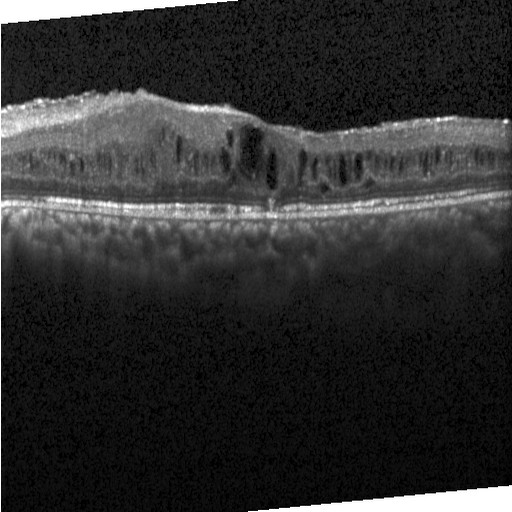 Heidelberg Spectralis. Through the macula. OCT B-scan — Diagnosis: diabetic macular edema (DME).